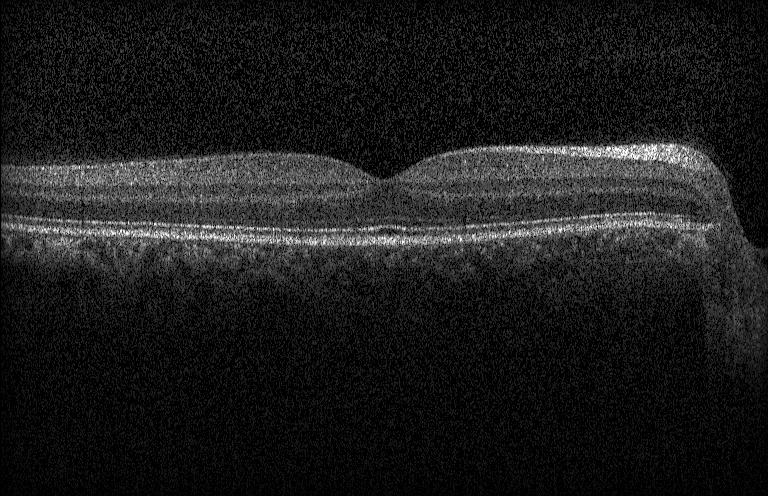

Neither choroidal neovascularization, diabetic macular edema, nor drusen.